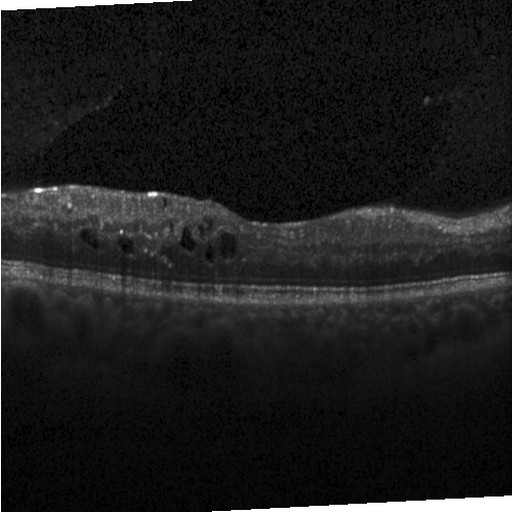

Retinal OCT cross-section showing DME.